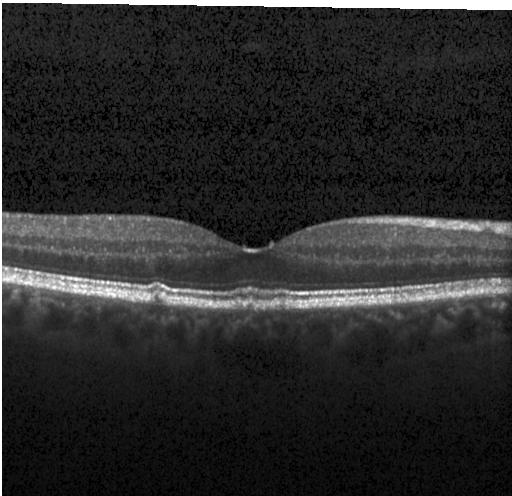

Spectral-domain OCT B-scan: multiple drusen.